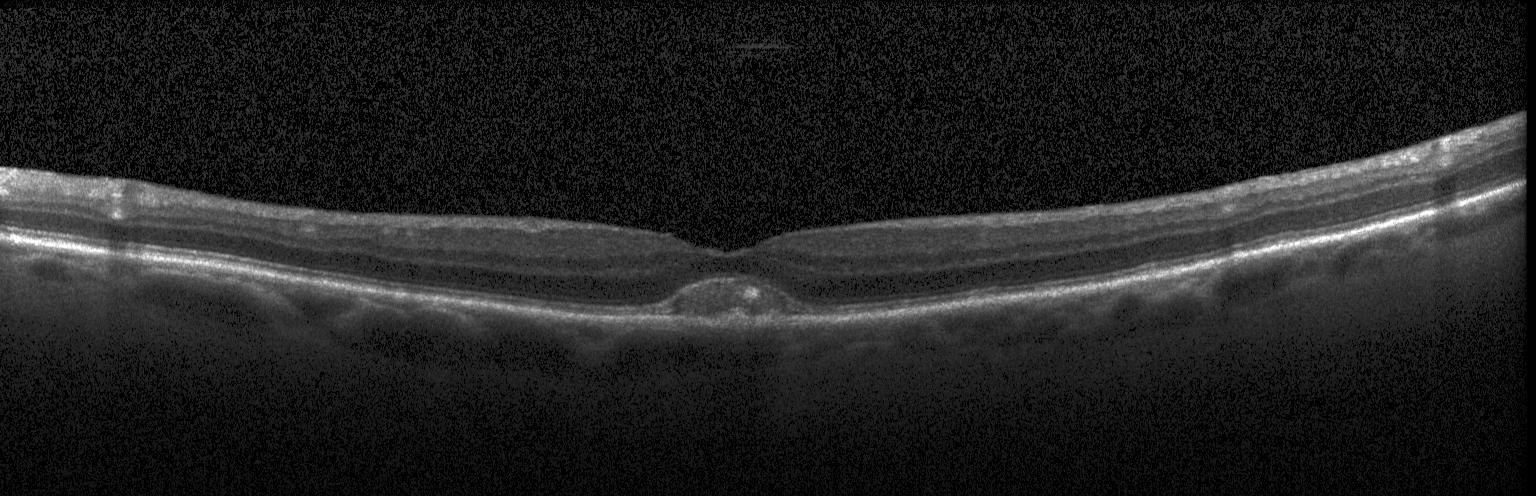

Acquired on a Heidelberg Spectralis. Spectral-domain OCT. Macular scan. Optical coherence tomography scan
Assessment: a choroidal neovascular membrane.